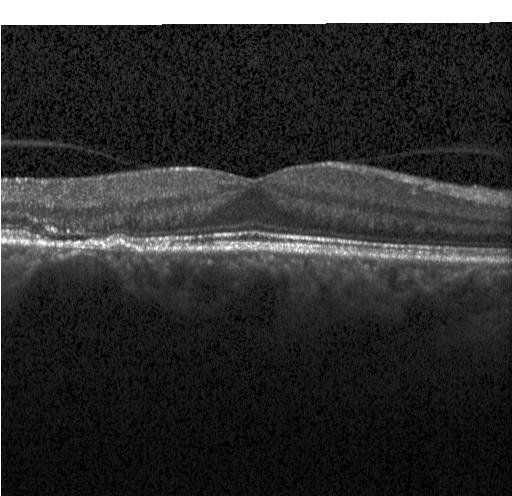

Spectral-domain OCT B-scan: a choroidal neovascular membrane.